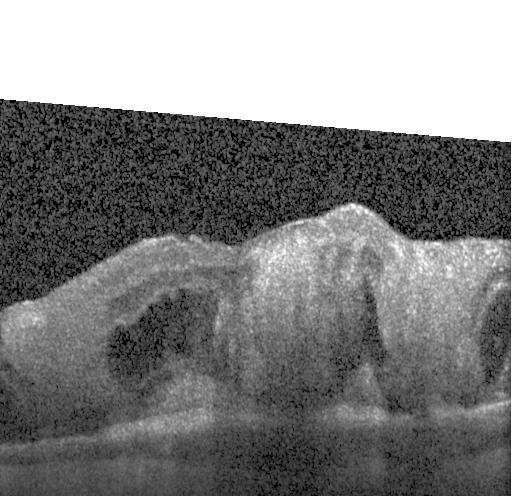
Diagnosis: a choroidal neovascular membrane.